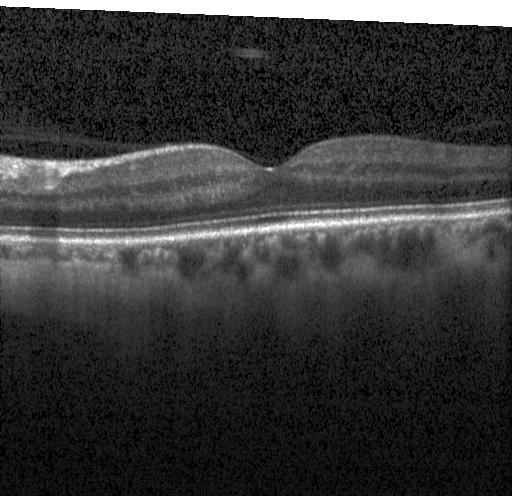

OCT line scan.
Macular OCT: neither choroidal neovascularization, diabetic macular edema, nor drusen.